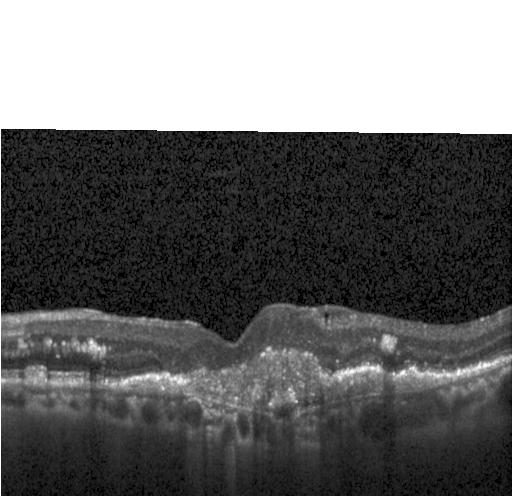
Heidelberg Spectralis OCT system, optical coherence tomography B-scan
Impression: choroidal neovascularization.